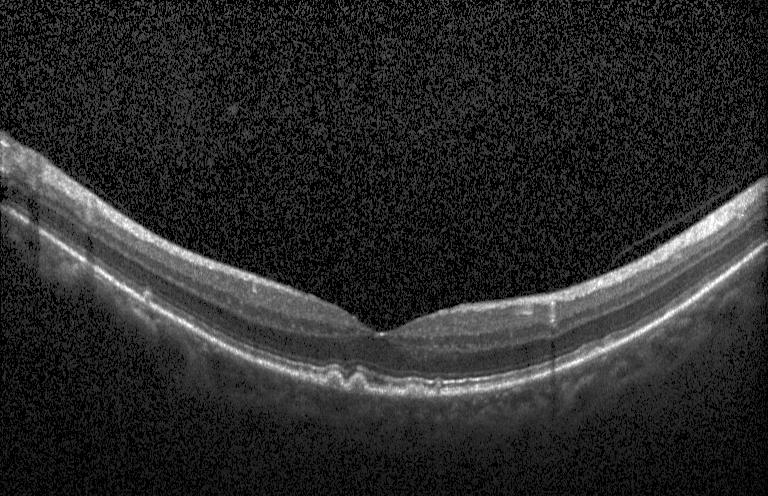
Spectral-domain optical coherence tomography · retinal OCT B-scan · horizontal scan through the fovea · acquired on a Heidelberg Spectralis
Dx: sub-RPE drusenoid deposits.